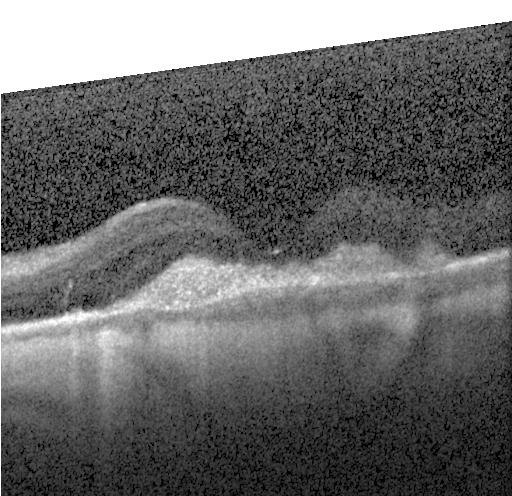
OCT scan showing a choroidal neovascular membrane.